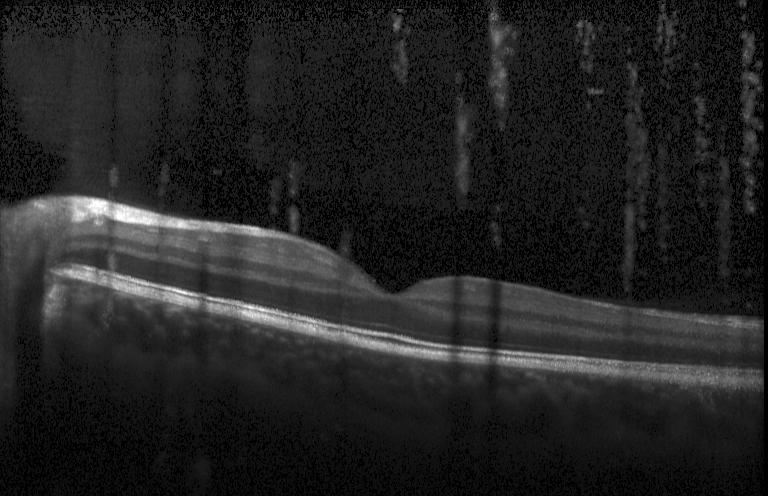
OCT line scan — Dx: neither choroidal neovascularization, diabetic macular edema, nor drusen.